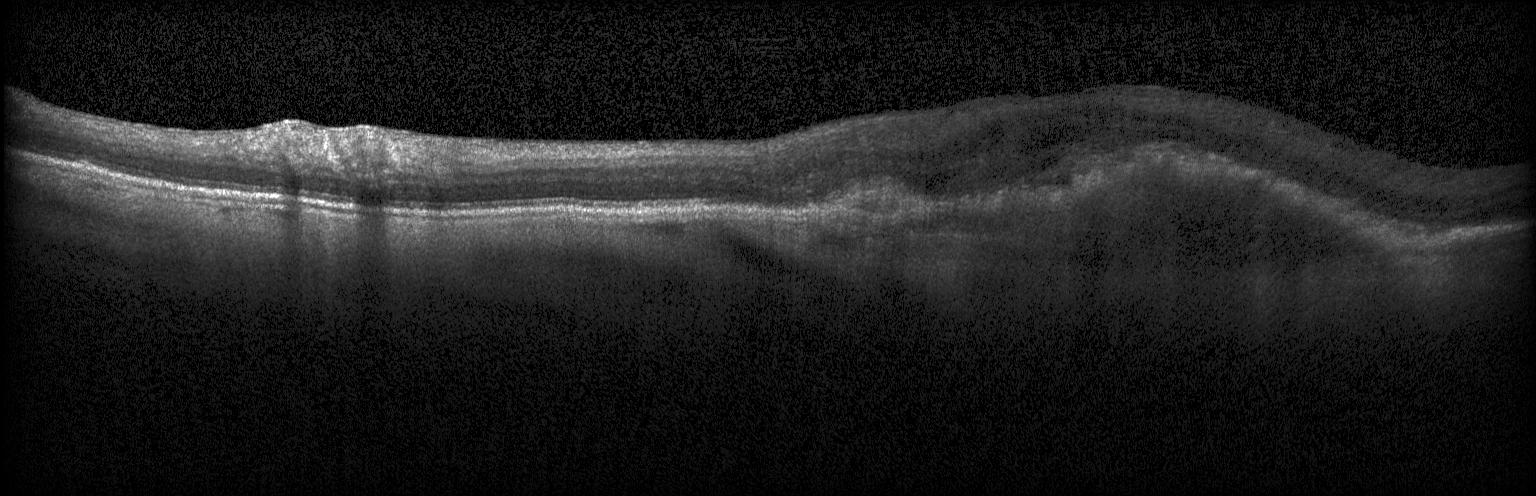
Macular OCT demonstrating a choroidal neovascular membrane.